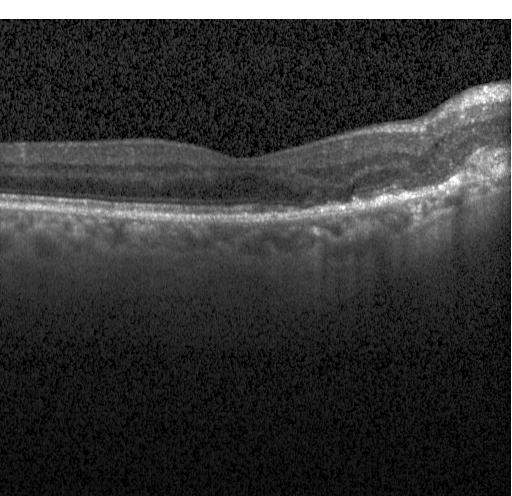
OCT B-scan.
Finding: CNV.